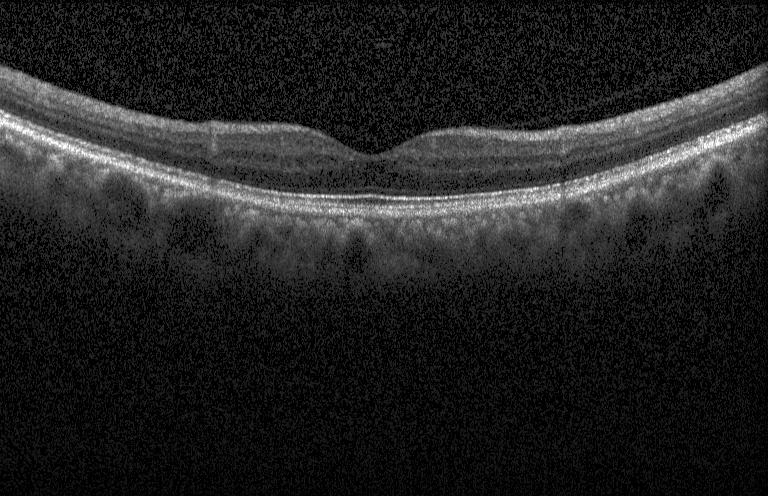

Macular OCT demonstrating neither CNV, DME, nor drusen.